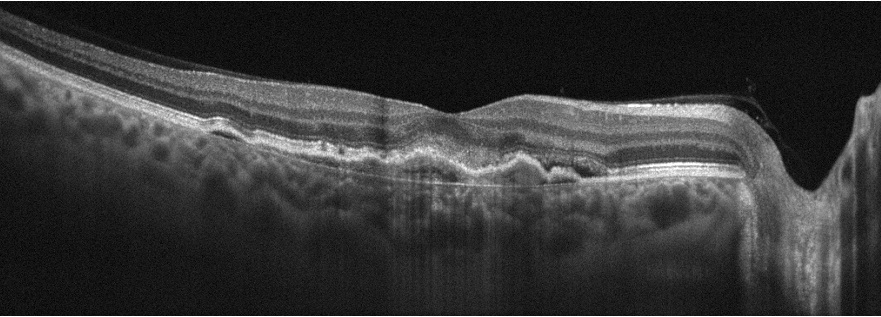

Optical coherence tomography scan
Diagnosis: AMD.